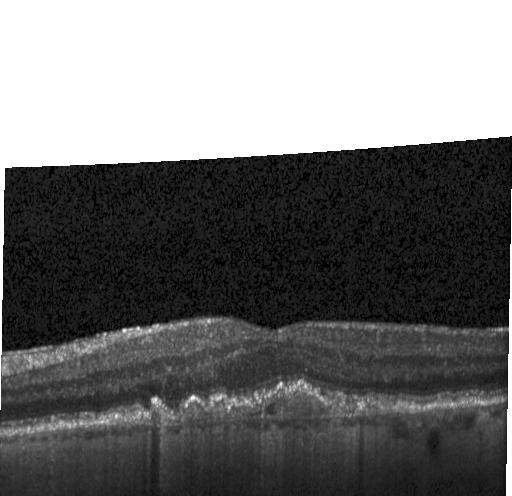
Horizontal scan through the fovea. OCT line scan.
Choroidal neovascularization (CNV).